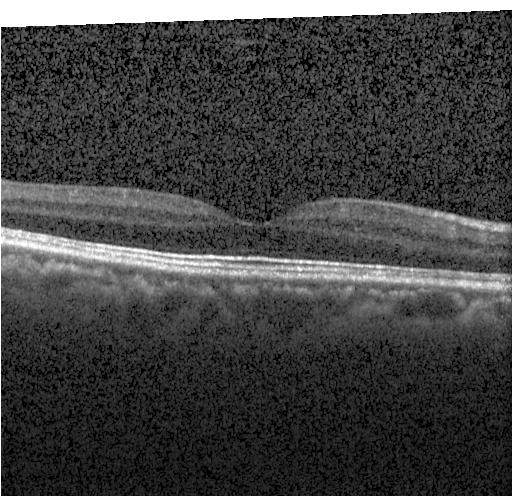 Dx: no choroidal neovascularization, no diabetic macular edema, and no drusen.